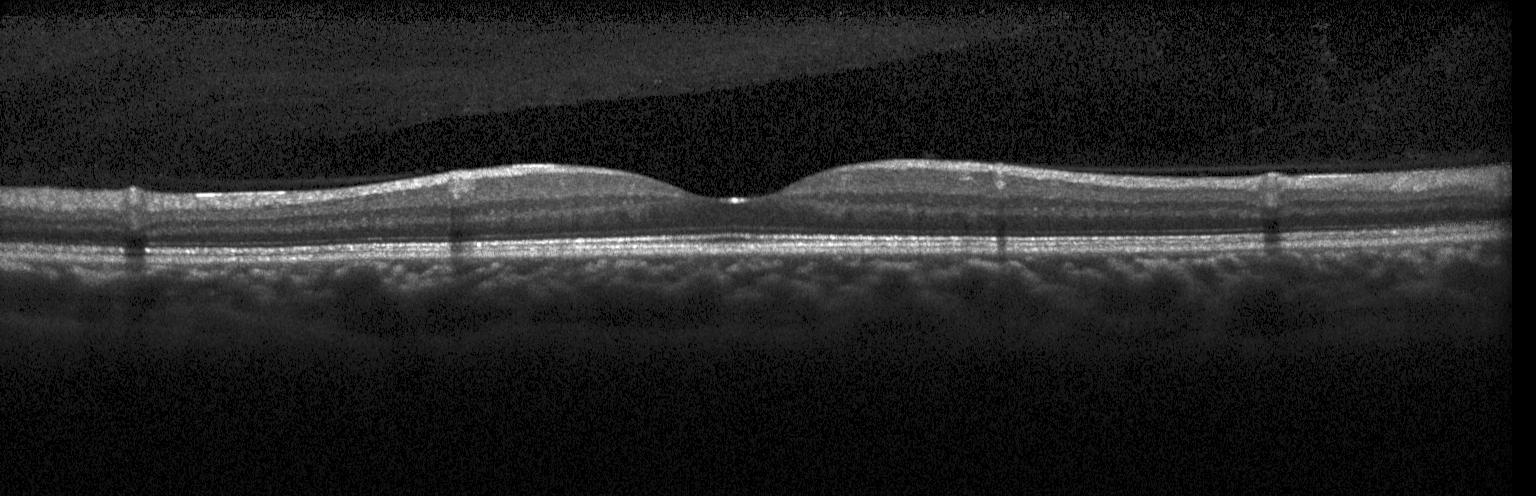

Dx: neither CNV, DME, nor drusen.